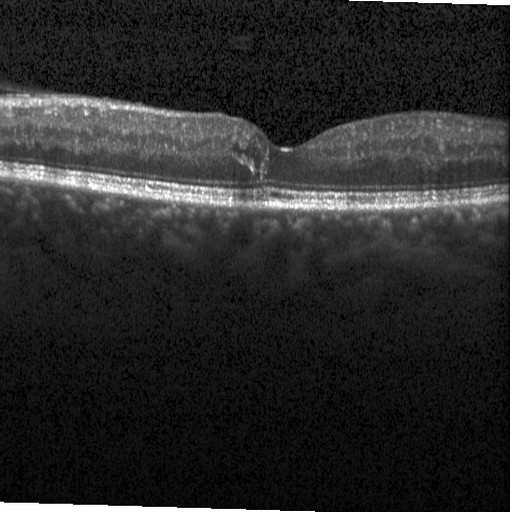
Diagnosis: diabetic macular edema (DME).